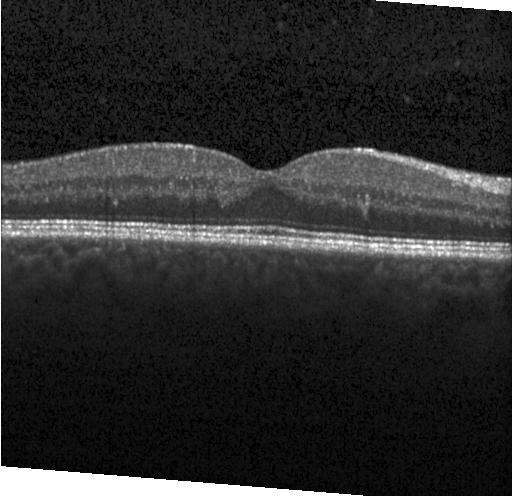 The scan shows neither choroidal neovascularization, diabetic macular edema, nor drusen.